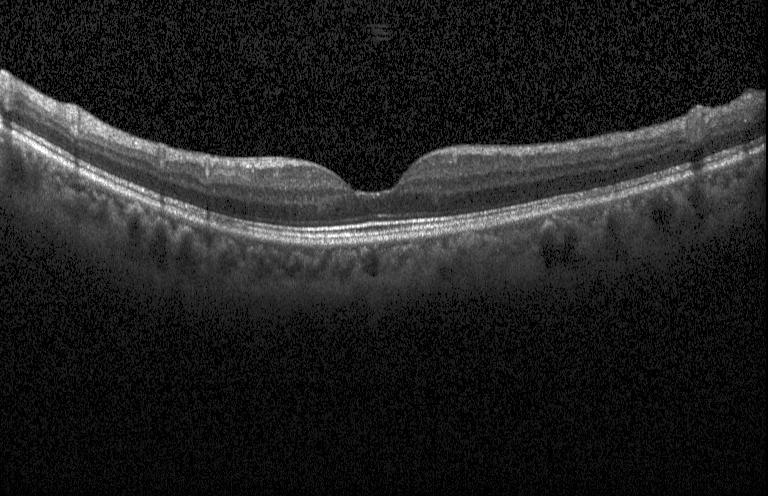 Macular scan, spectral-domain OCT, instrument: Heidelberg Spectralis, retinal OCT B-scan
Impression: no choroidal neovascularization, diabetic macular edema, or drusen.